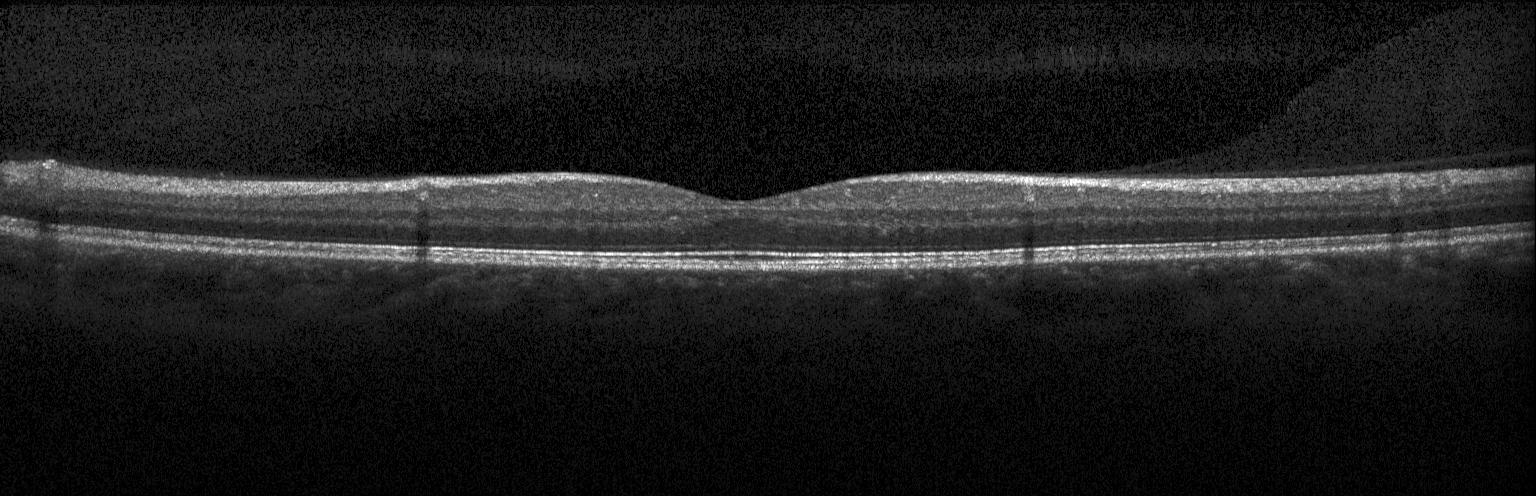 Acquired on a Heidelberg Spectralis · fovea-centered · retinal OCT B-scan.
Assessment: no choroidal neovascularization, diabetic macular edema, or drusen.